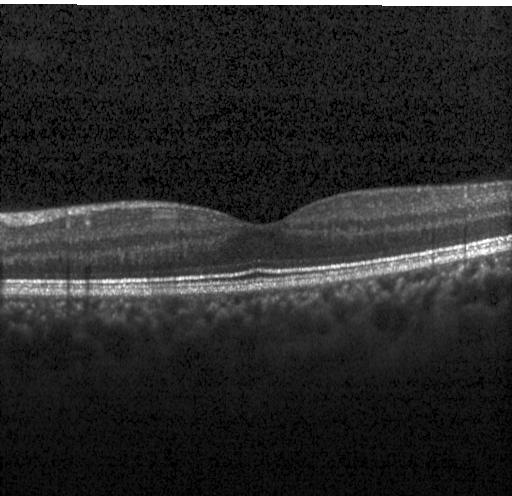 OCT scan showing neither choroidal neovascularization, diabetic macular edema, nor drusen.